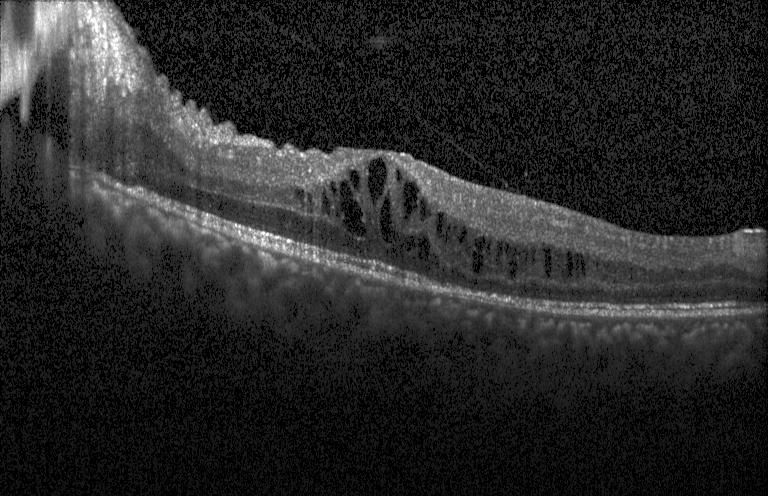

Spectral-domain optical coherence tomography. Optical coherence tomography B-scan — Finding: diabetic macular edema.